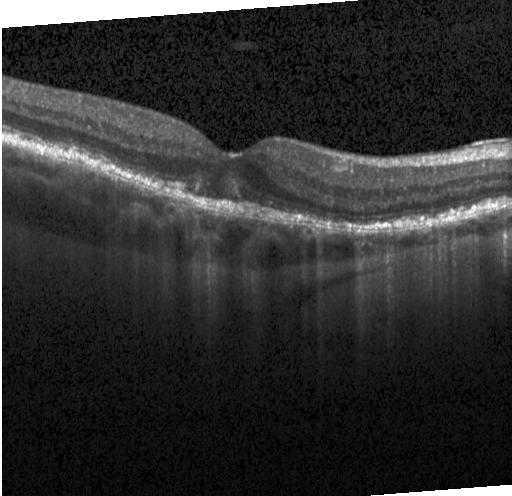

Optical coherence tomography B-scan
Assessment: choroidal neovascularization.